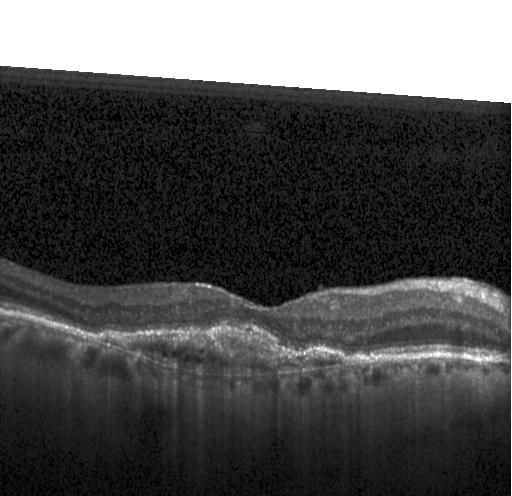
Retinal OCT B-scan. OCT finding: a choroidal neovascular membrane.